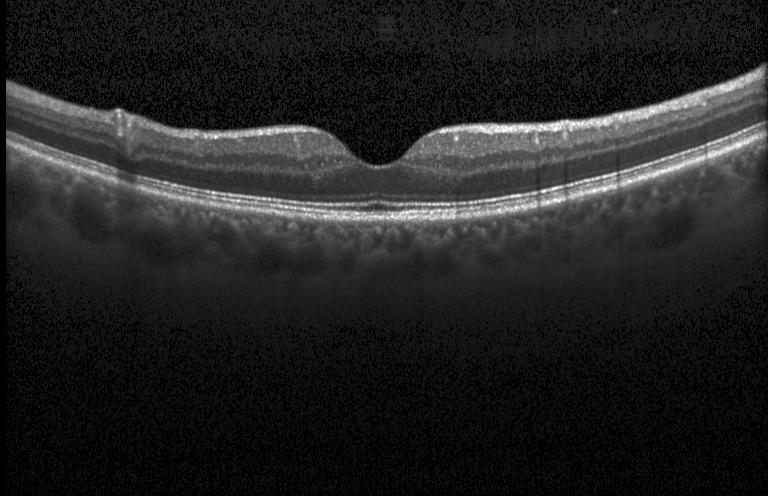

This B-scan demonstrates no evidence of choroidal neovascularization, diabetic macular edema, or drusen.